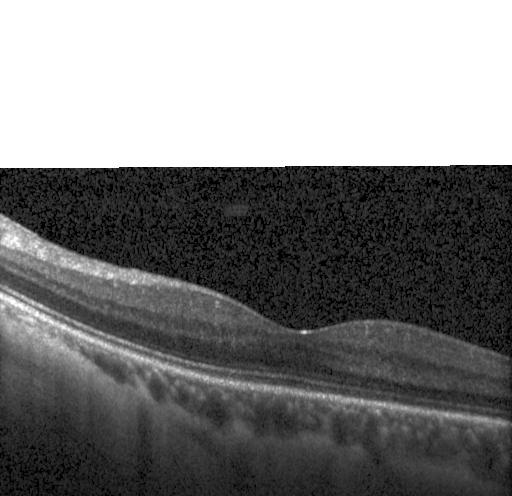
Dx: neither choroidal neovascularization, diabetic macular edema, nor drusen.